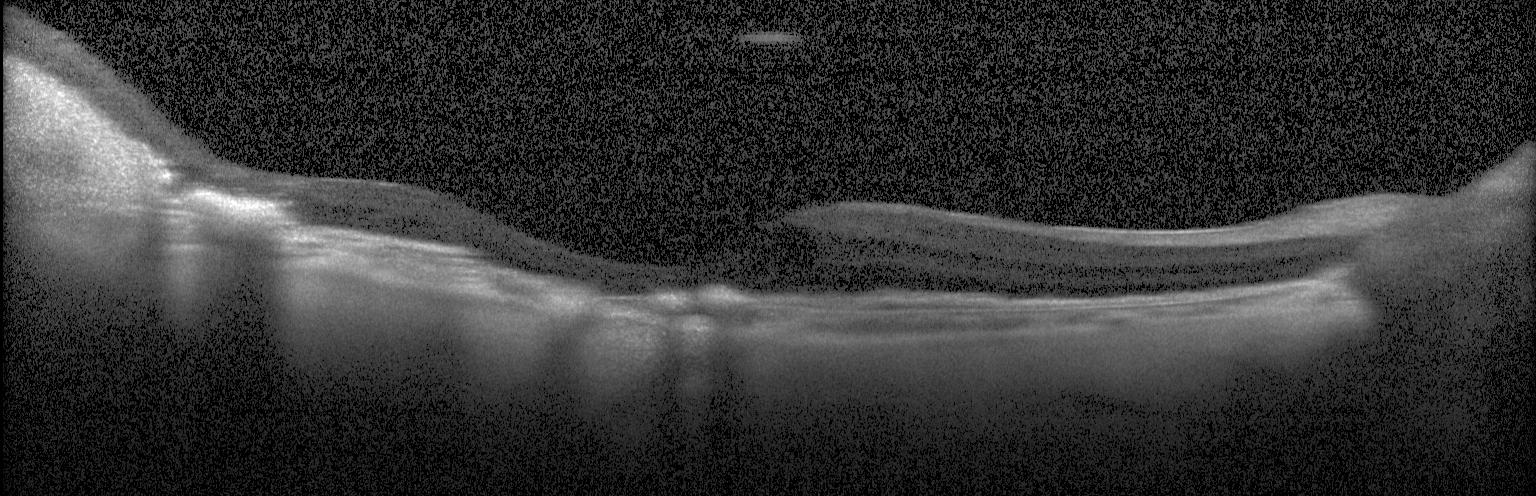

Assessment: a choroidal neovascular membrane.